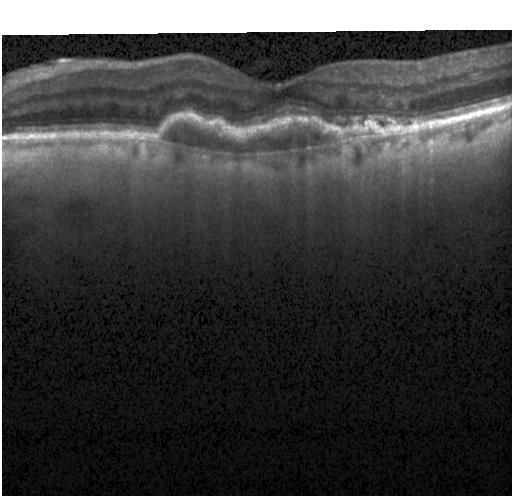 Spectral-domain OCT, macular scan, optical coherence tomography scan
The scan shows a choroidal neovascular membrane.